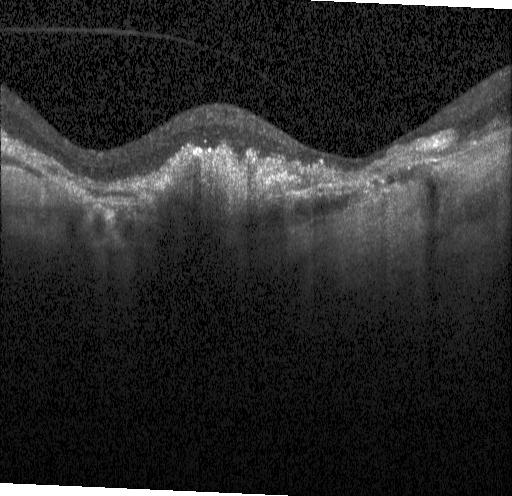

Through the macula; instrument: Heidelberg Spectralis; spectral-domain optical coherence tomography; optical coherence tomography scan.
Impression: a choroidal neovascular membrane.